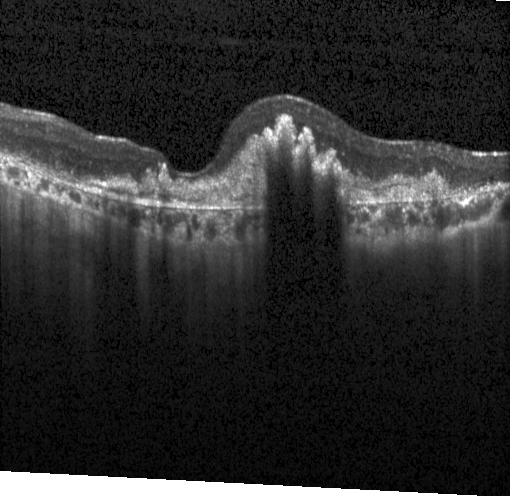

Finding: a choroidal neovascular membrane.